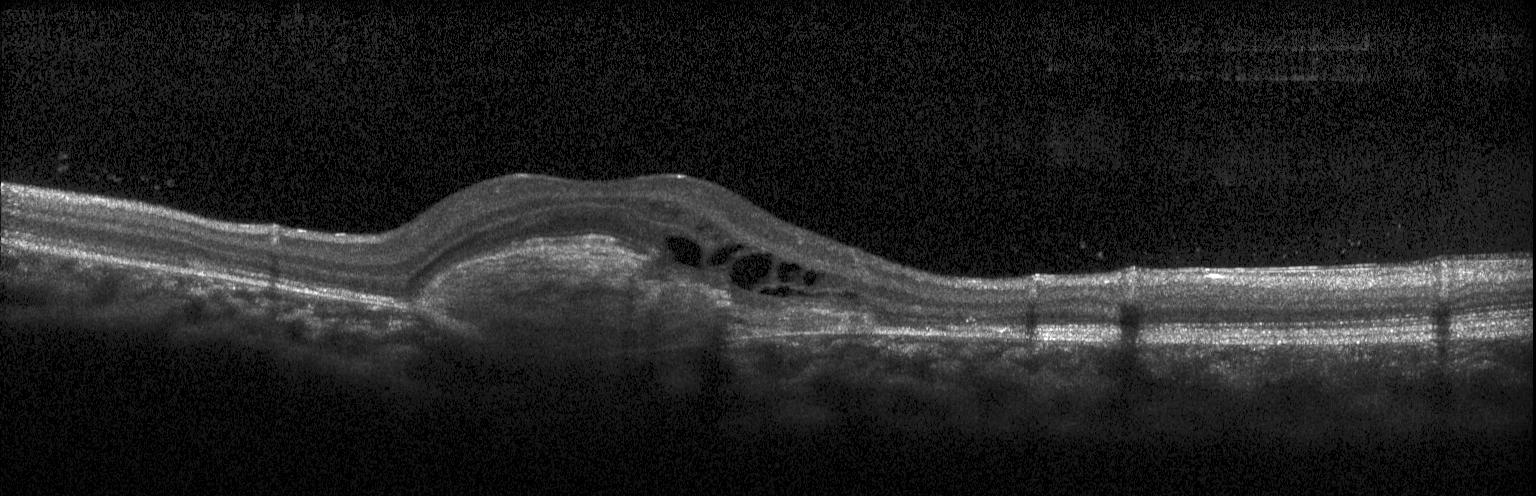
Dx: CNV.